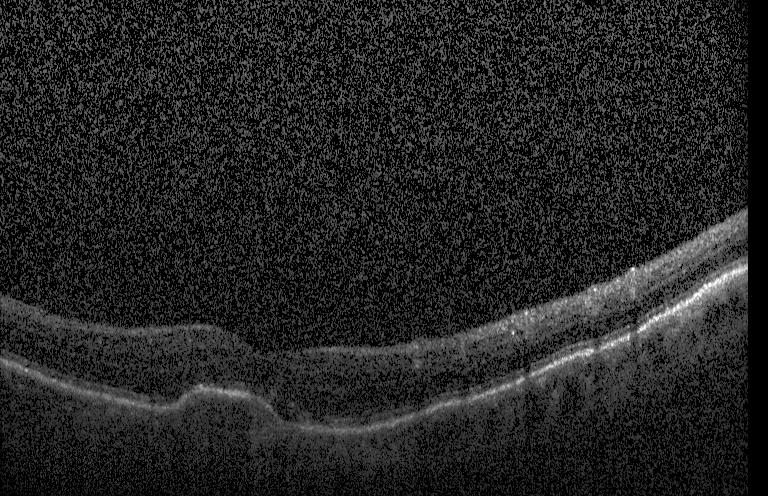
SD-OCT; optical coherence tomography scan. Finding: choroidal neovascularization (CNV).